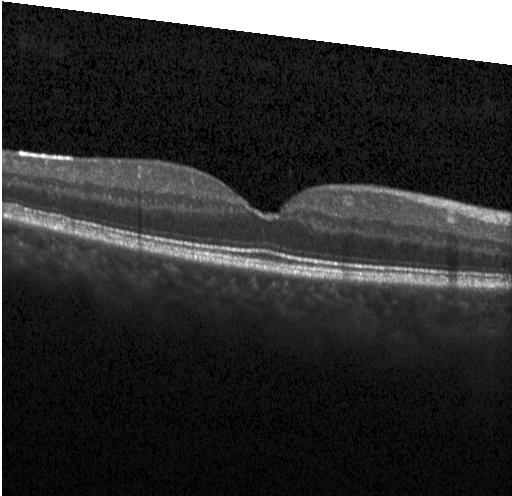
Heidelberg Spectralis OCT system, spectral-domain OCT, retinal OCT cross-section, fovea-centered
Finding: neither choroidal neovascularization, diabetic macular edema, nor drusen.